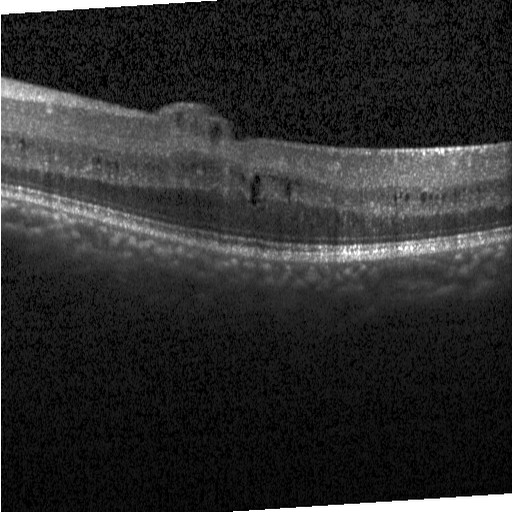

OCT B-scan — The scan shows DME.